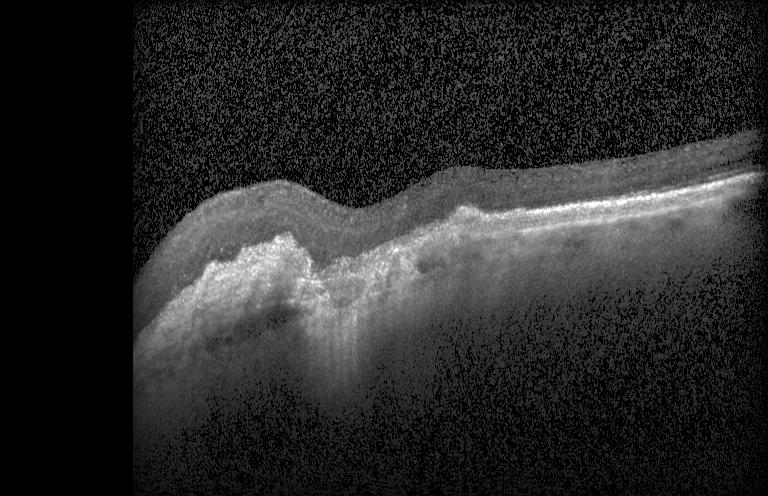 Spectral-domain OCT; Heidelberg Spectralis OCT system; OCT B-scan. Impression: a choroidal neovascular membrane.